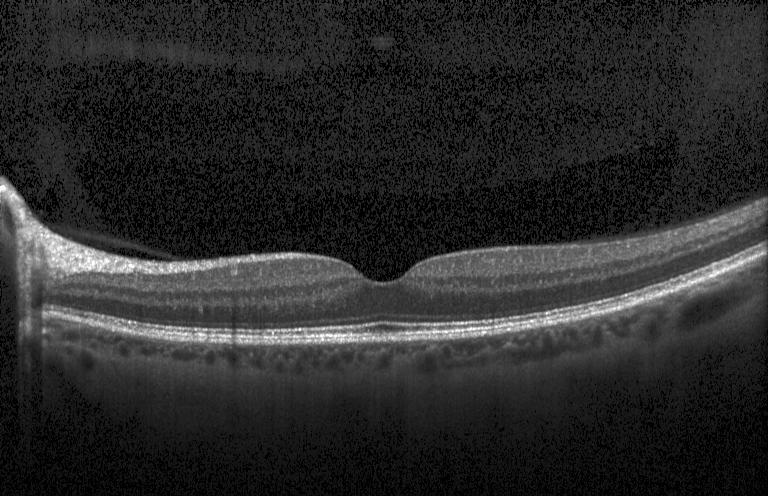
OCT line scan. Macular scan. Spectral-domain optical coherence tomography
Impression: no choroidal neovascularization, diabetic macular edema, or drusen.